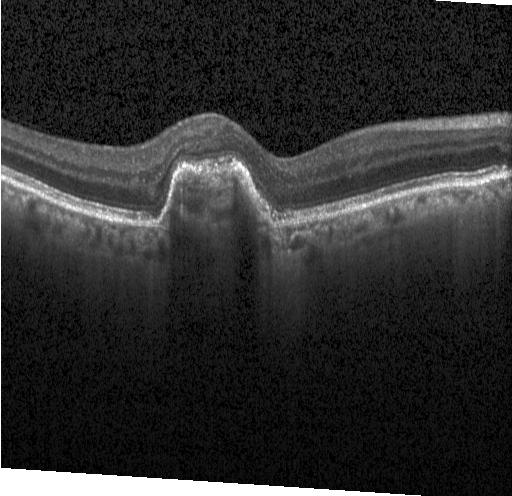
Heidelberg Spectralis; retinal OCT cross-section; through the macula.
Diagnosis: choroidal neovascularization (CNV).